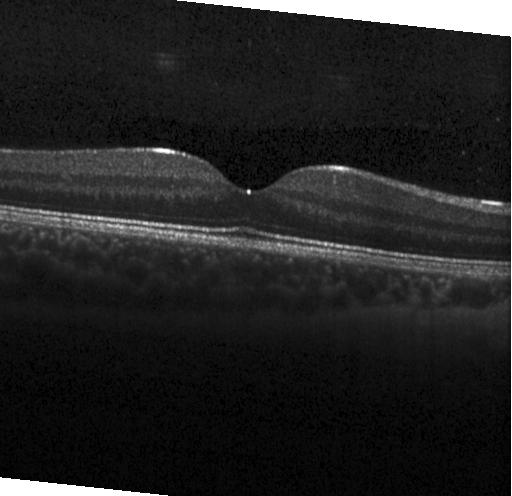 Optical coherence tomography B-scan. Finding: neither choroidal neovascularization, diabetic macular edema, nor drusen.